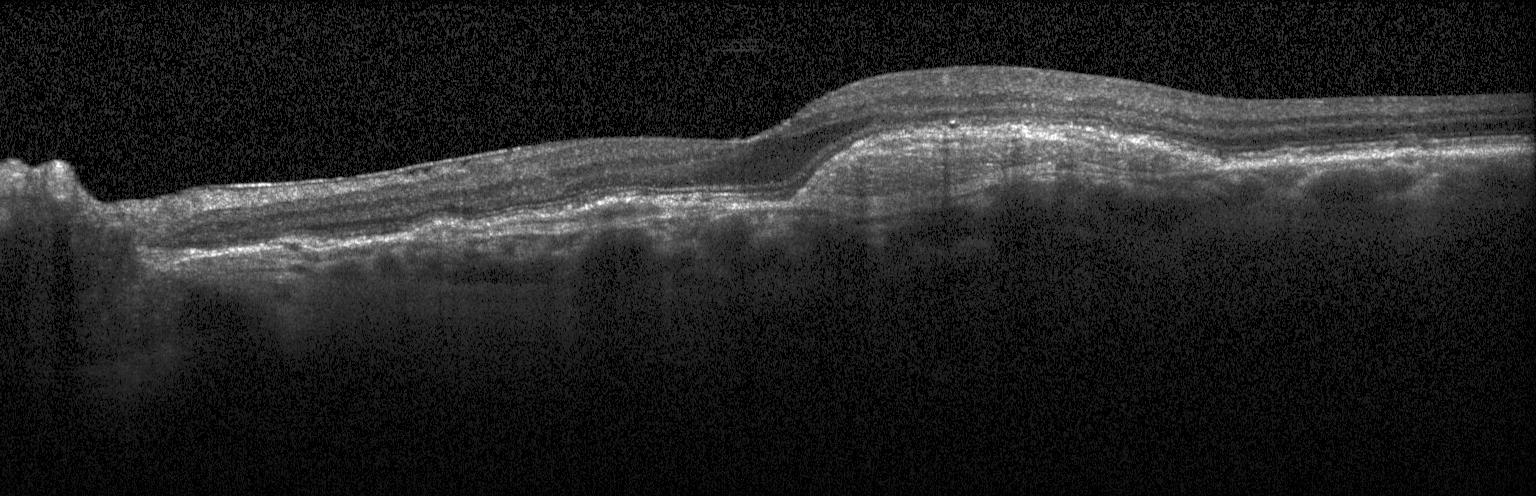 Spectral-domain OCT · centered on the fovea · OCT line scan · Heidelberg Spectralis OCT system
CNV.